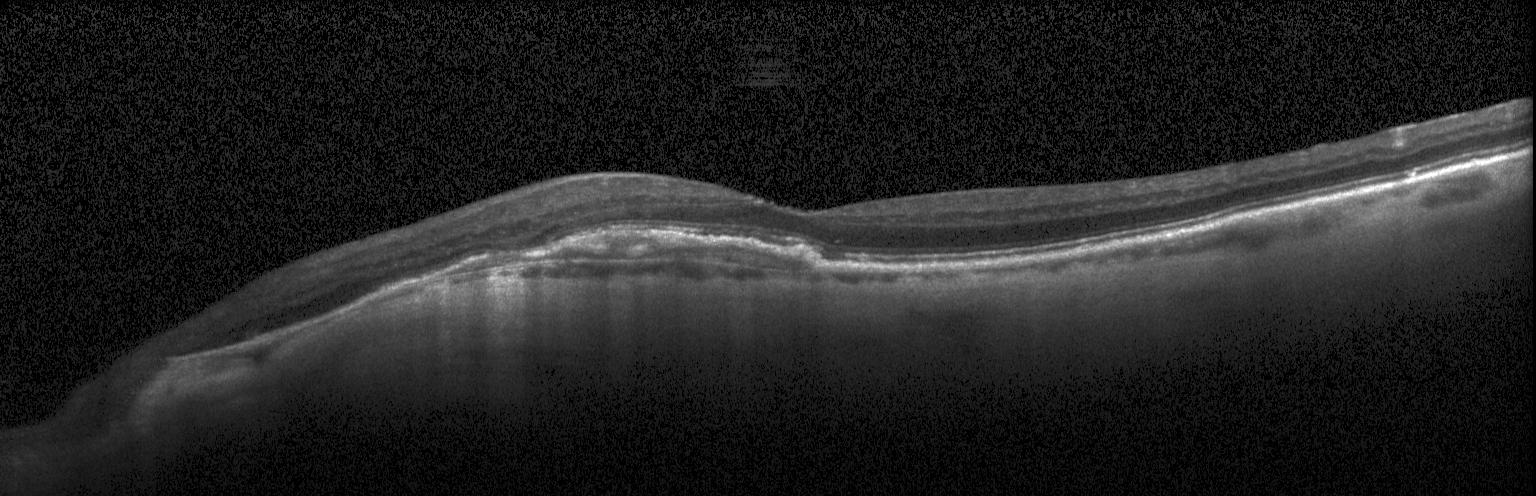
Finding: CNV.